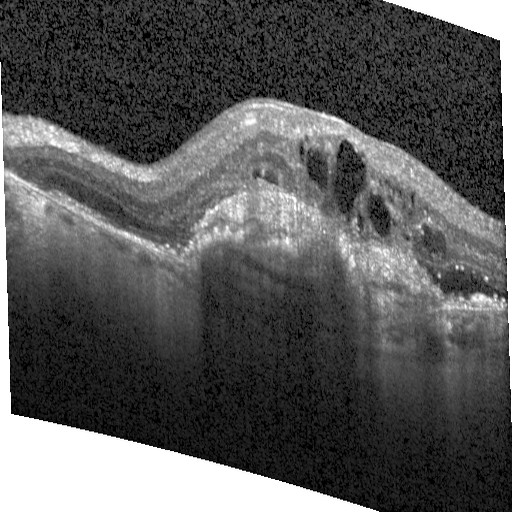

Heidelberg Spectralis OCT system; spectral-domain OCT; OCT B-scan; horizontal scan through the fovea
Dx: DME.